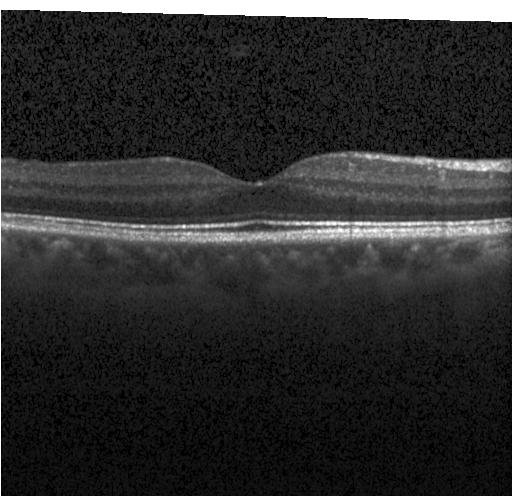
SD-OCT · Heidelberg Spectralis OCT system · OCT B-scan.
Macular OCT: neither choroidal neovascularization, diabetic macular edema, nor drusen.